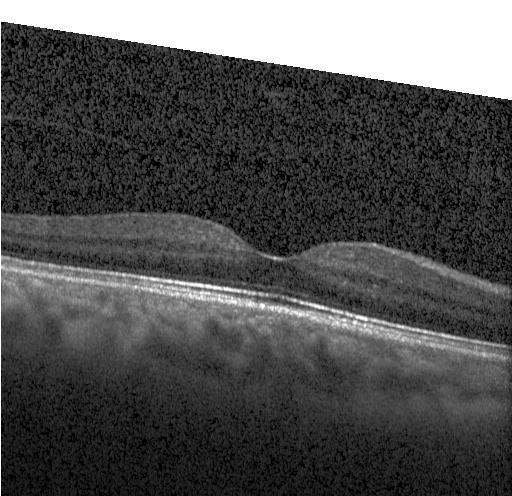 Macular OCT: no CNV, no DME, and no drusen.